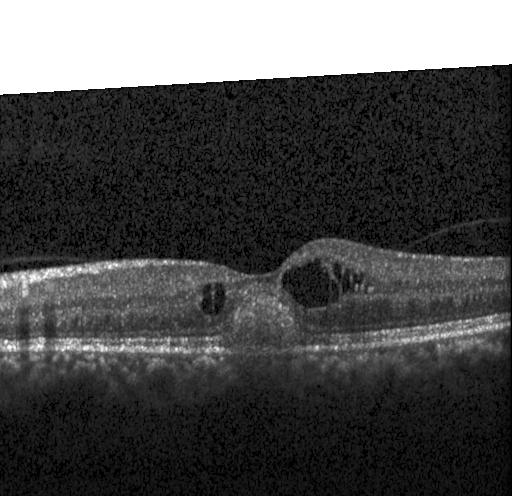
Macular scan. Retinal OCT B-scan — Diagnosis: a choroidal neovascular membrane.